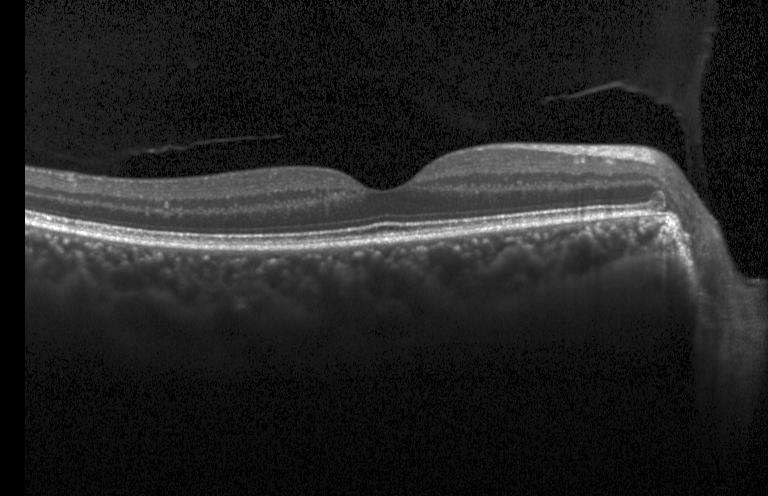 OCT finding: no choroidal neovascularization, no diabetic macular edema, and no drusen.